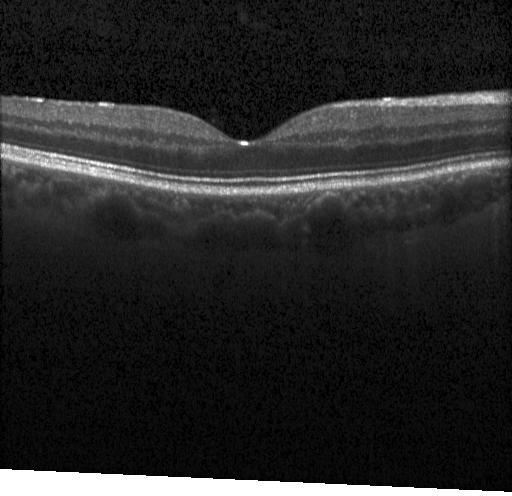 Spectral-domain OCT B-scan: no choroidal neovascularization, diabetic macular edema, or drusen.